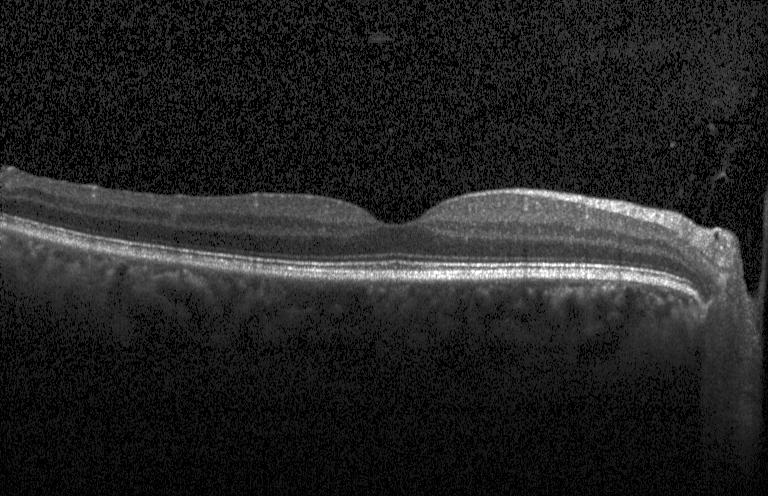 Impression: no choroidal neovascularization, no diabetic macular edema, and no drusen.